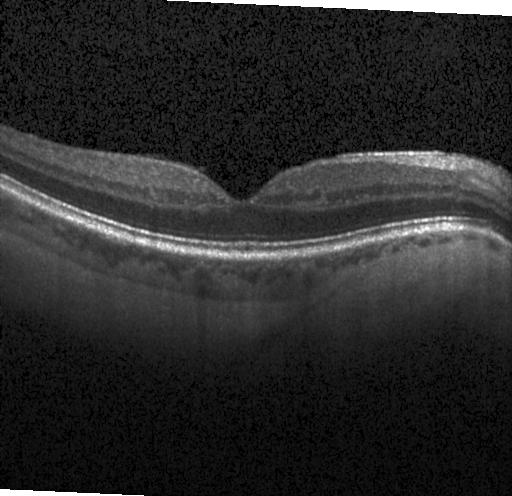

Finding: no choroidal neovascularization, diabetic macular edema, or drusen.